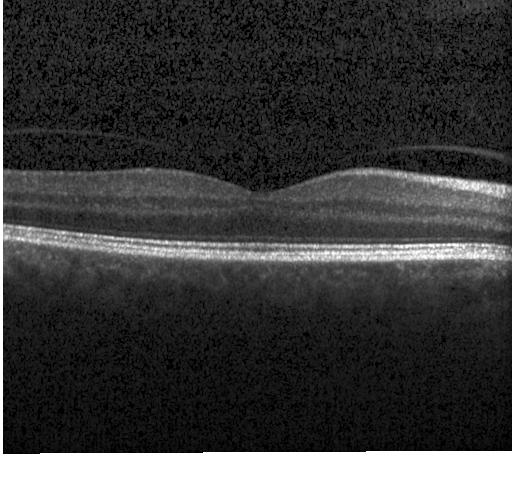
OCT B-scan; fovea-centered; spectral-domain OCT; Heidelberg Spectralis. Impression: neither choroidal neovascularization, diabetic macular edema, nor drusen.